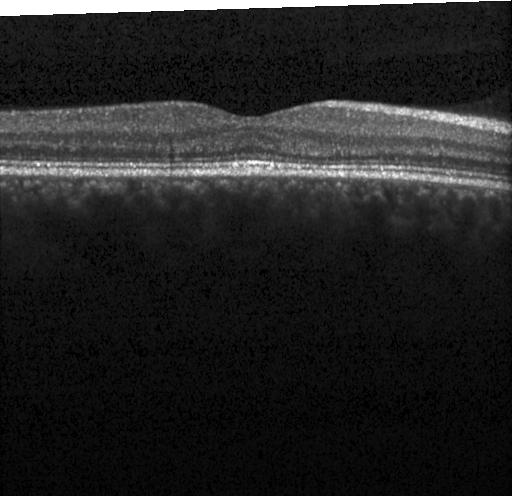
OCT B-scan, spectral-domain optical coherence tomography — Assessment: no evidence of choroidal neovascularization, diabetic macular edema, or drusen.